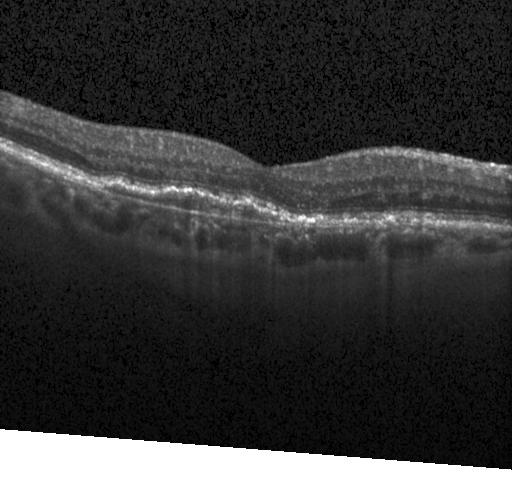 Finding: a choroidal neovascular membrane.